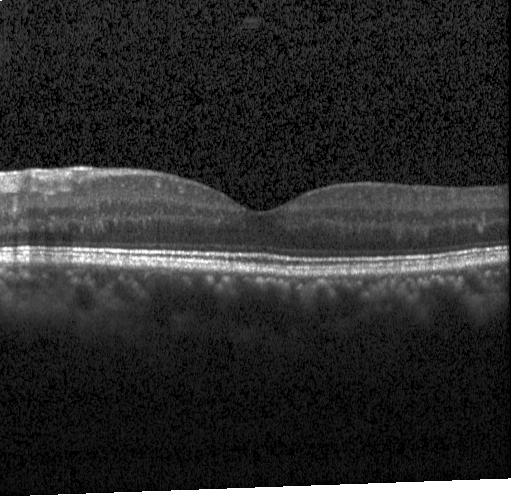

Macular OCT: no choroidal neovascularization, no diabetic macular edema, and no drusen.